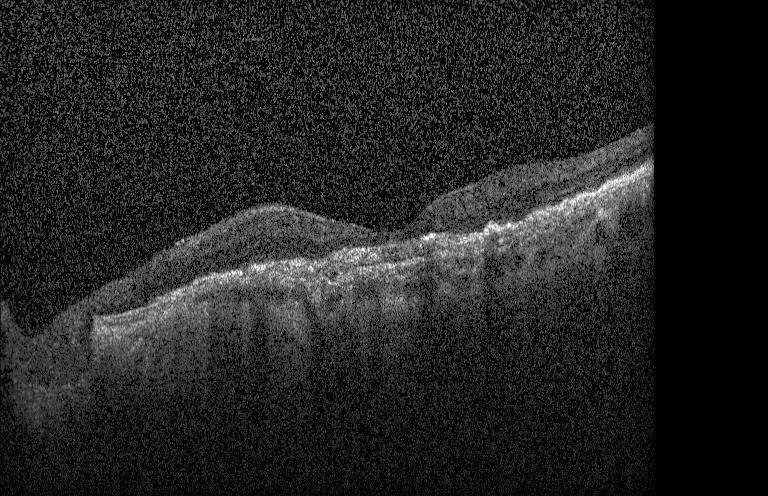

Finding: choroidal neovascularization.